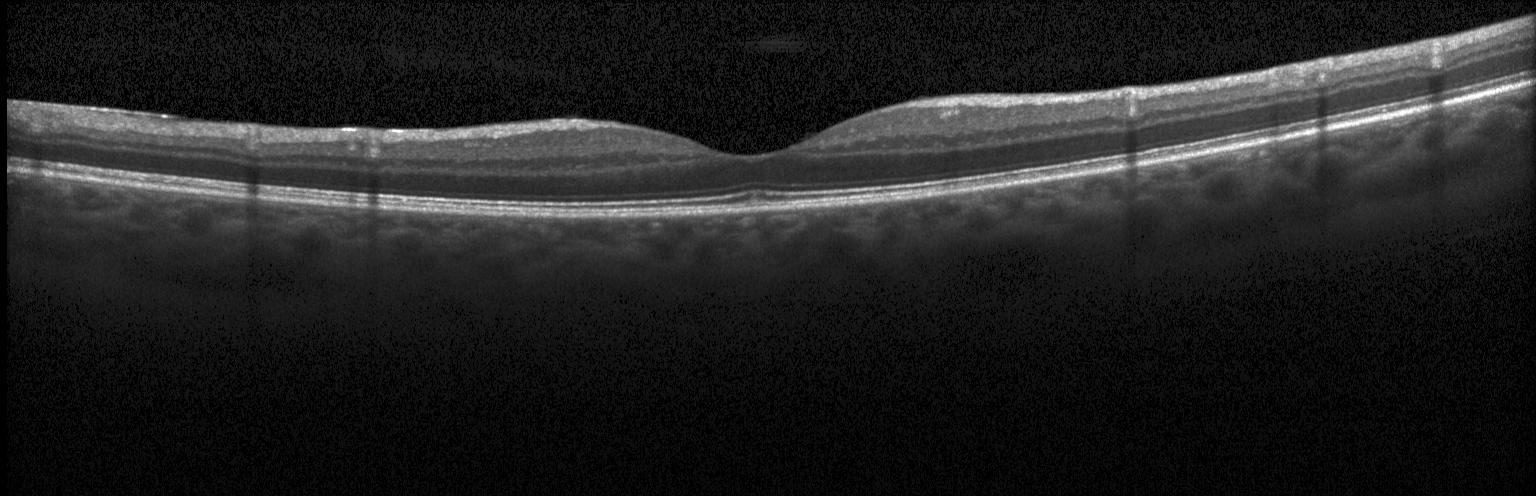
Diagnosis: no evidence of choroidal neovascularization, diabetic macular edema, or drusen.